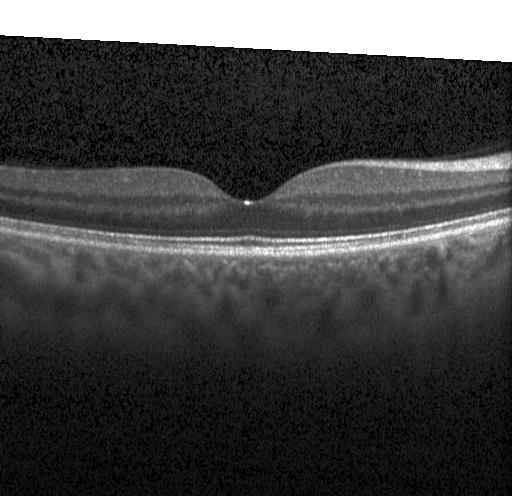 OCT finding: no evidence of CNV, DME, or drusen.